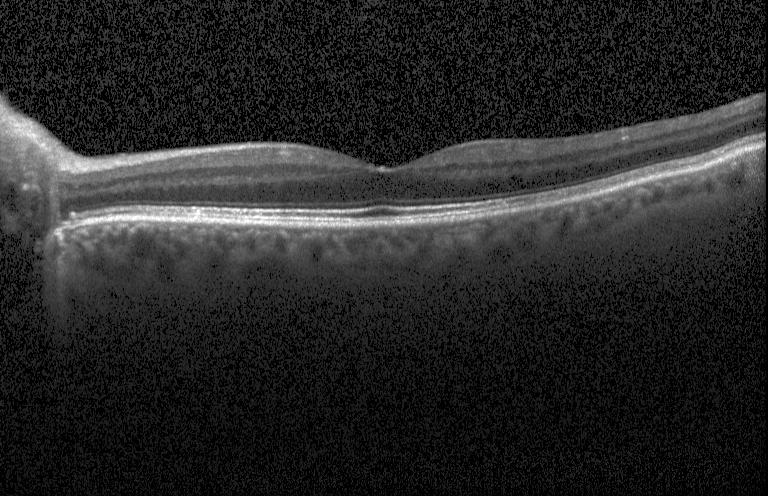
Heidelberg Spectralis, spectral-domain OCT, retinal OCT B-scan — Finding: no choroidal neovascularization, no diabetic macular edema, and no drusen.